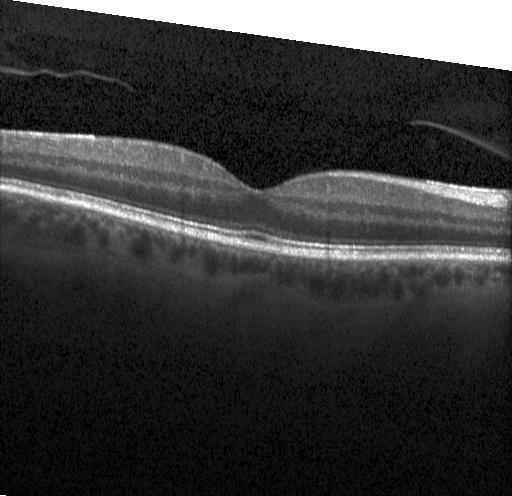
Impression: neither choroidal neovascularization, diabetic macular edema, nor drusen.